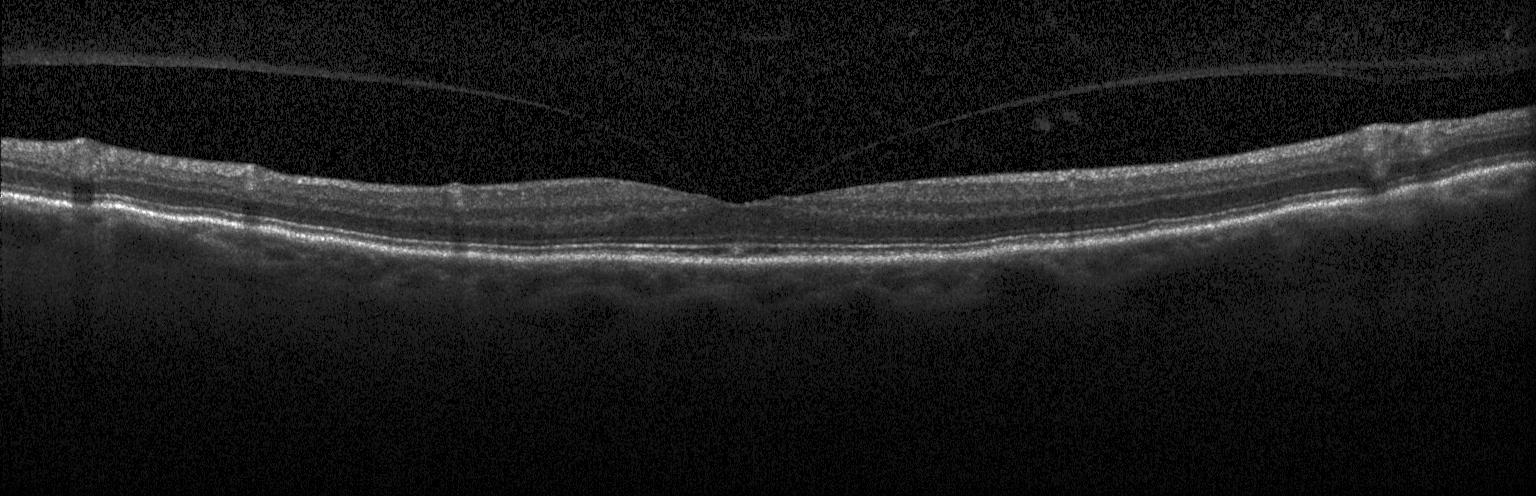

Heidelberg Spectralis · macular scan · retinal OCT B-scan · SD-OCT
Macular OCT: no choroidal neovascularization, no diabetic macular edema, and no drusen.